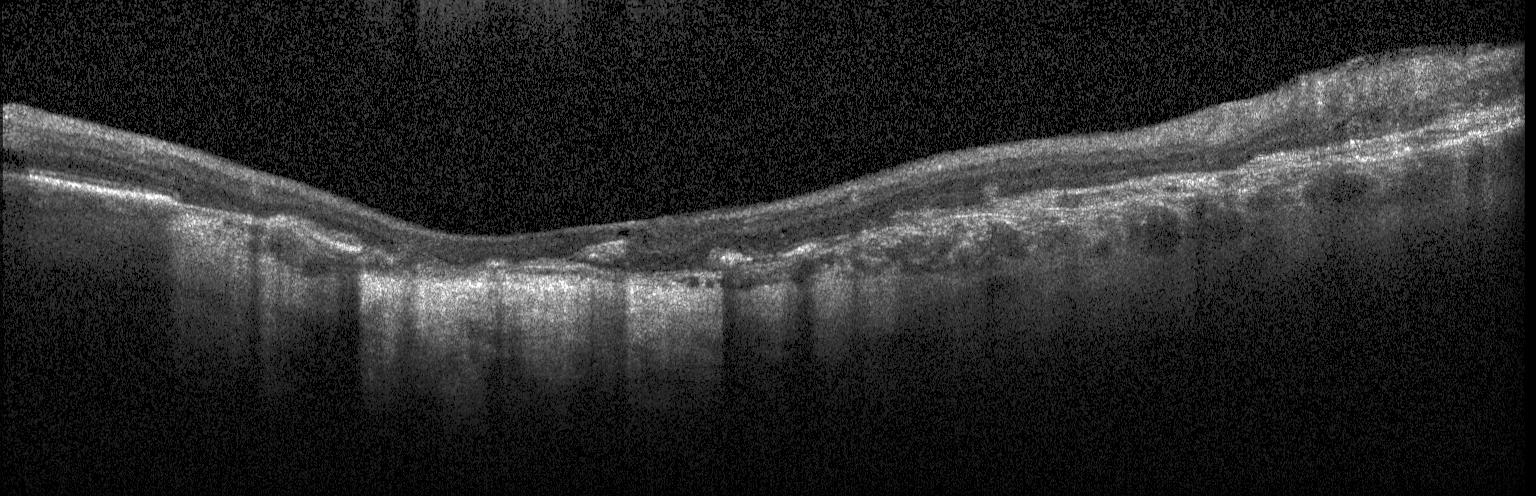

Optical coherence tomography scan — Dx: a choroidal neovascular membrane.